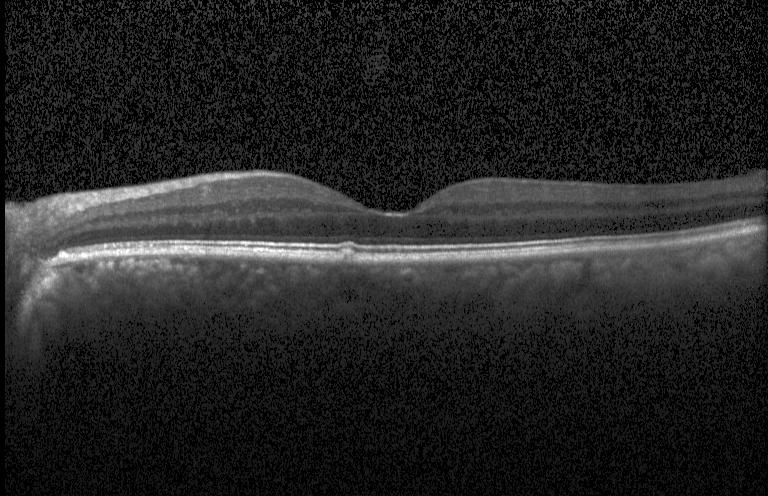
Spectral-domain OCT B-scan: no evidence of CNV, DME, or drusen.